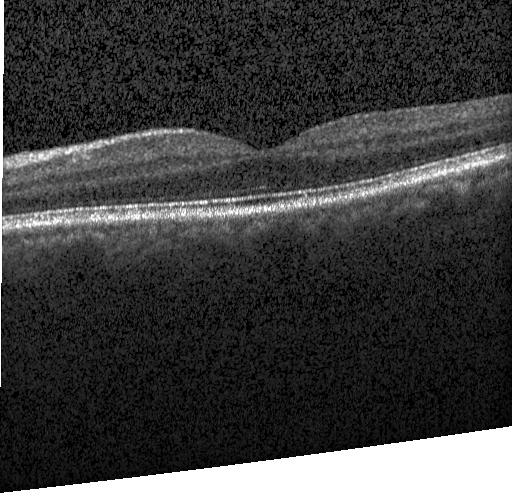 Optical coherence tomography scan.
Diagnosis: no evidence of choroidal neovascularization, diabetic macular edema, or drusen.